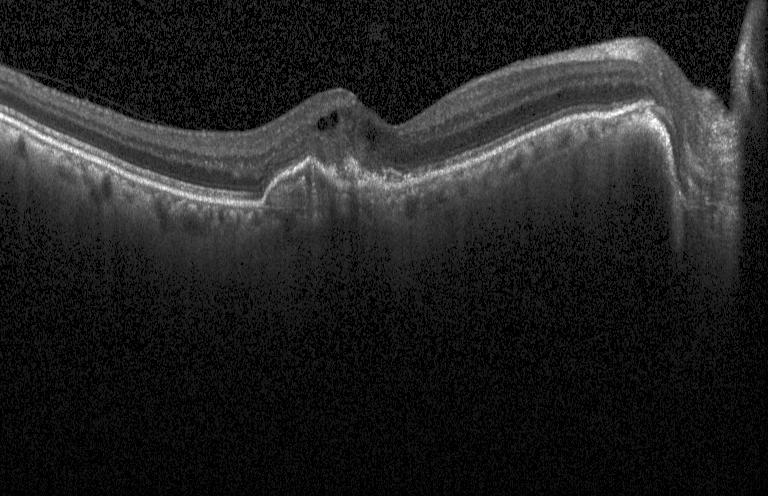
Optical coherence tomography scan.
Finding: choroidal neovascularization (CNV).